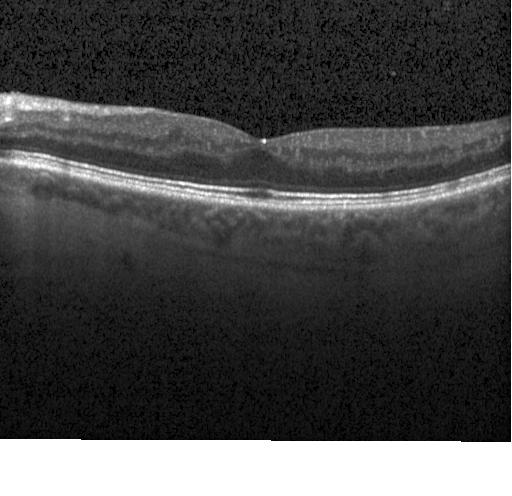

Heidelberg Spectralis. Optical coherence tomography scan
Dx: neither choroidal neovascularization, diabetic macular edema, nor drusen.